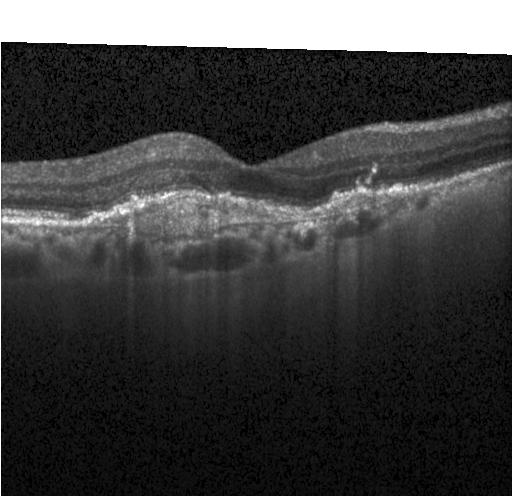

The scan shows a choroidal neovascular membrane.